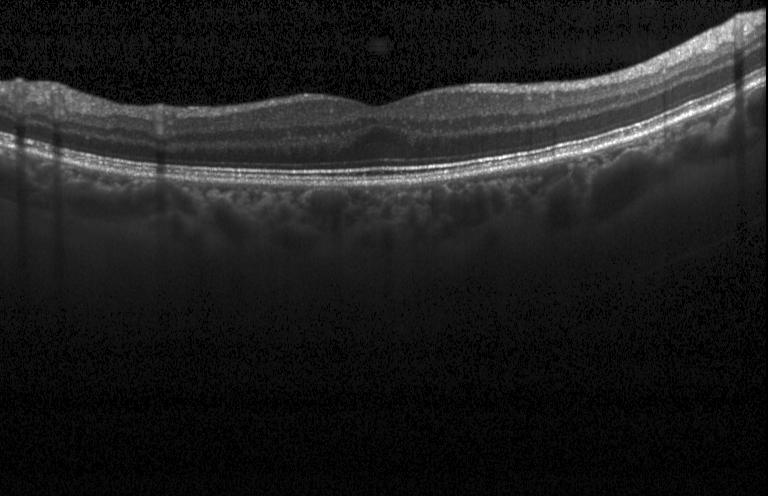

Spectral-domain OCT B-scan: no CNV, DME, or drusen.